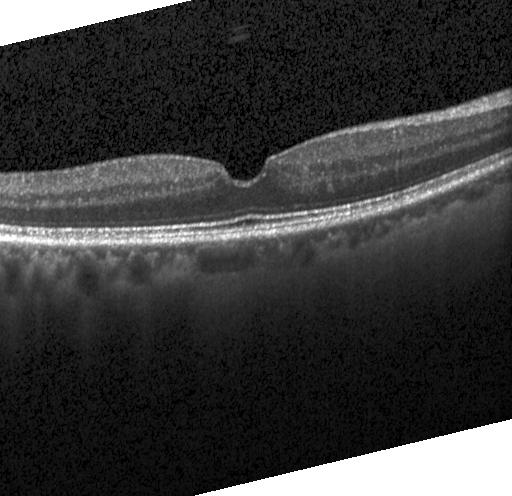
Diagnosis: no choroidal neovascularization, diabetic macular edema, or drusen.